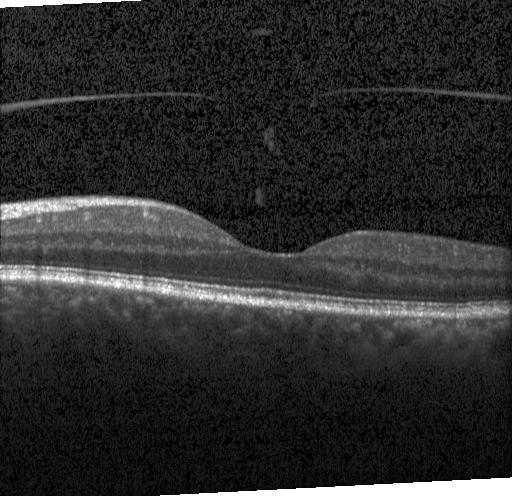 OCT B-scan. Finding: no evidence of CNV, DME, or drusen.